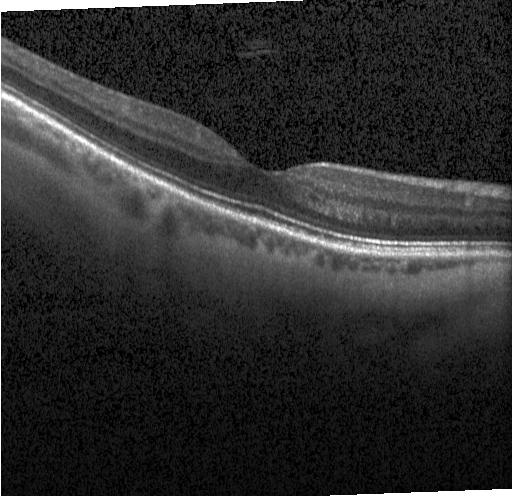
Heidelberg Spectralis OCT system · retinal OCT B-scan · spectral-domain optical coherence tomography · through the macula
This B-scan demonstrates no CNV, no DME, and no drusen.